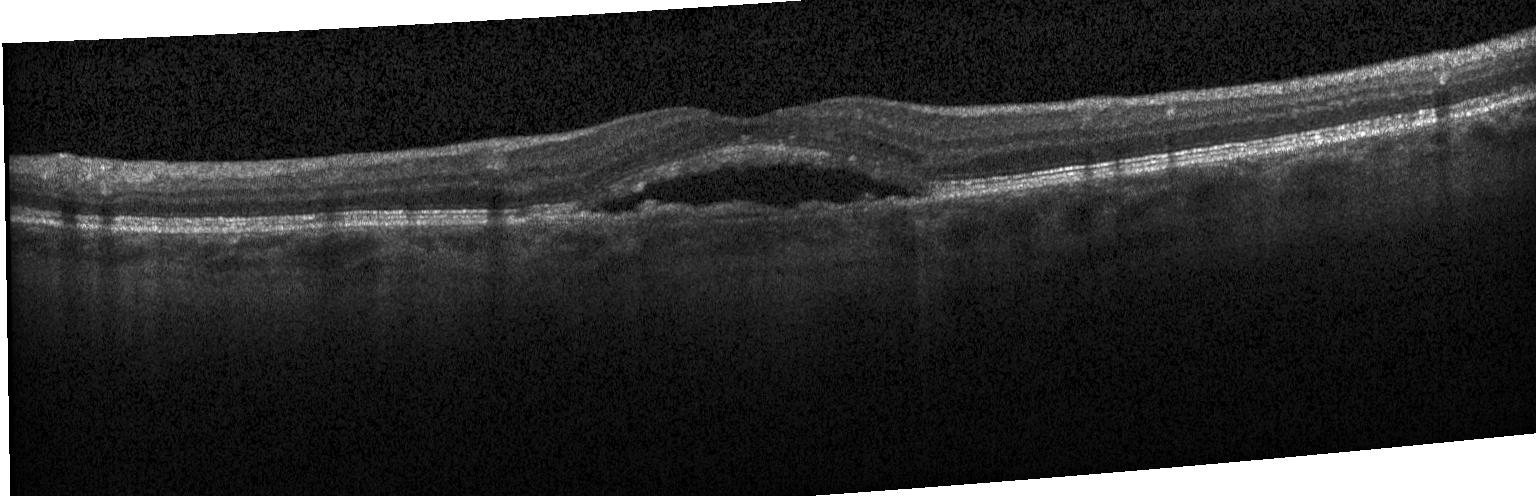

Diagnosis: choroidal neovascularization.